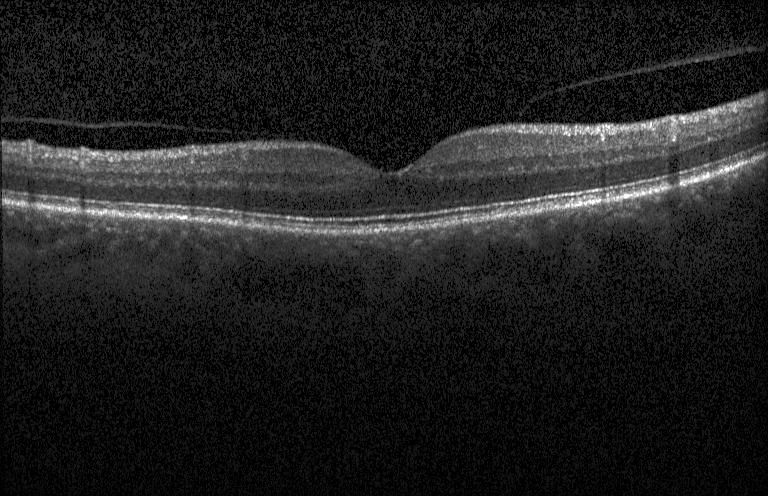

OCT finding: no choroidal neovascularization, diabetic macular edema, or drusen.